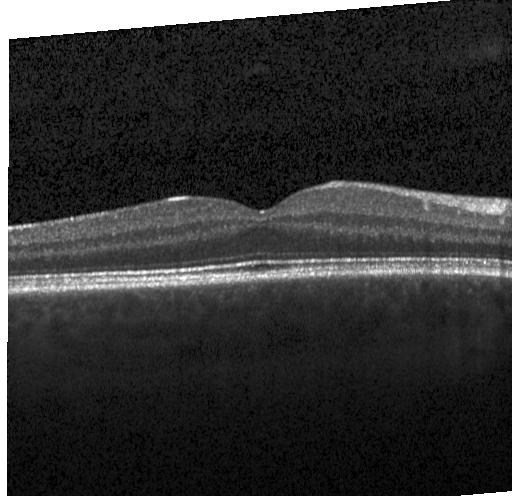

Optical coherence tomography scan; spectral-domain OCT. Diagnosis: no choroidal neovascularization, no diabetic macular edema, and no drusen.